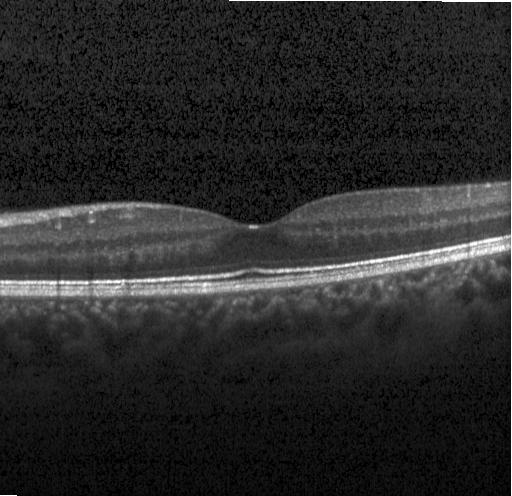
OCT finding: neither choroidal neovascularization, diabetic macular edema, nor drusen.